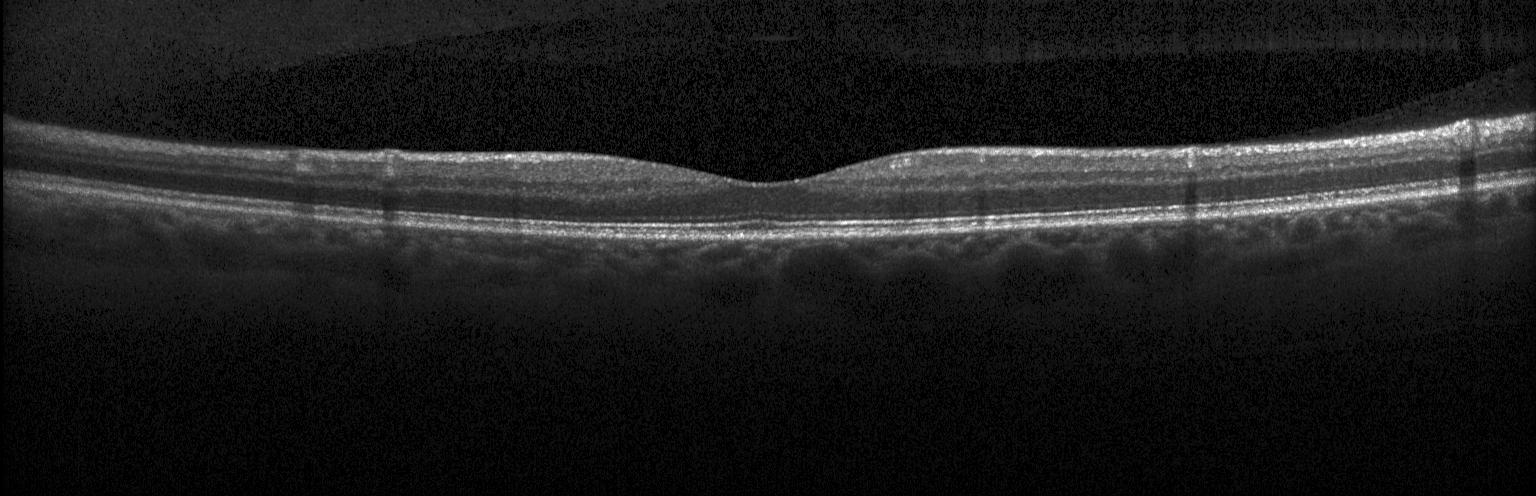
Horizontal scan through the fovea · acquired on a Heidelberg Spectralis · spectral-domain optical coherence tomography · optical coherence tomography scan. This B-scan demonstrates neither choroidal neovascularization, diabetic macular edema, nor drusen.